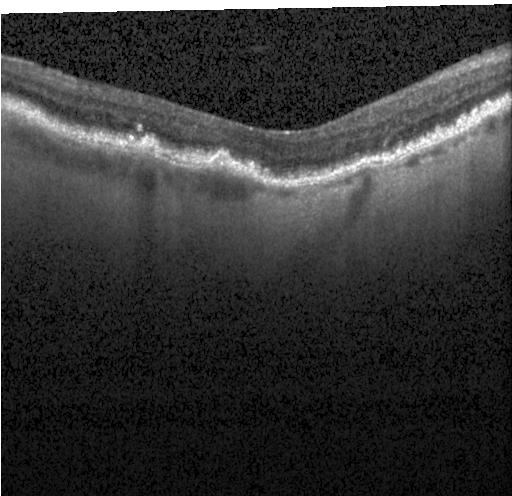 Assessment: a choroidal neovascular membrane.